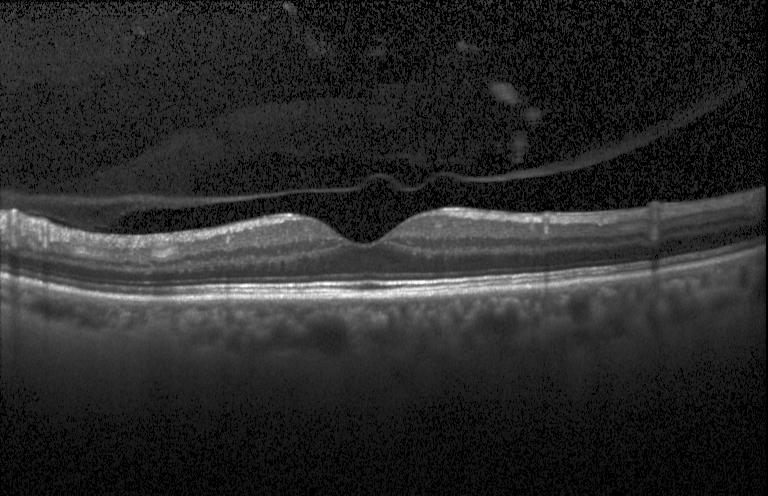
Retinal OCT cross-section — No CNV, no DME, and no drusen.